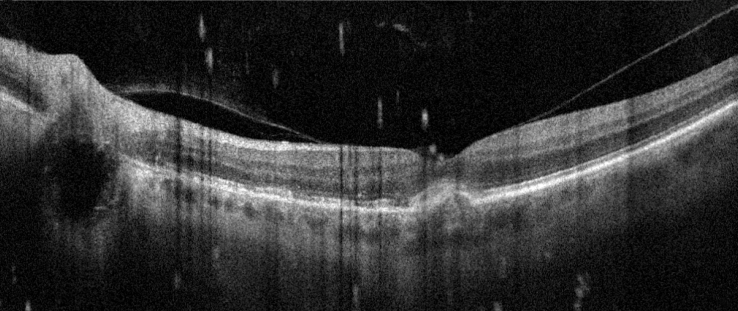
Macular OCT: AMD.